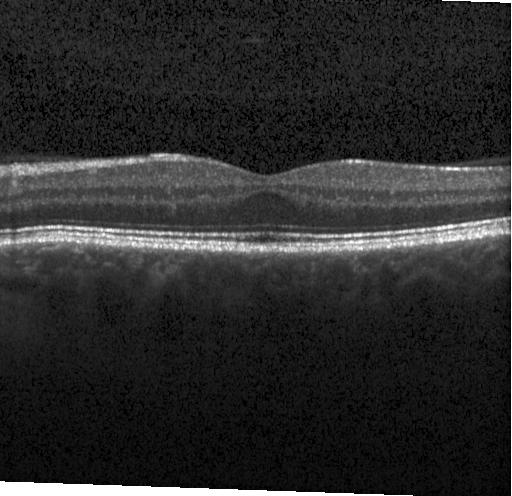 OCT line scan, macular scan, spectral-domain optical coherence tomography.
Diagnosis: no CNV, DME, or drusen.